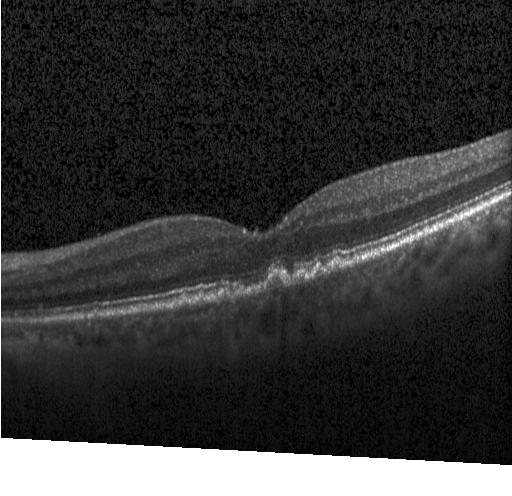 Spectral-domain OCT B-scan: multiple drusen.